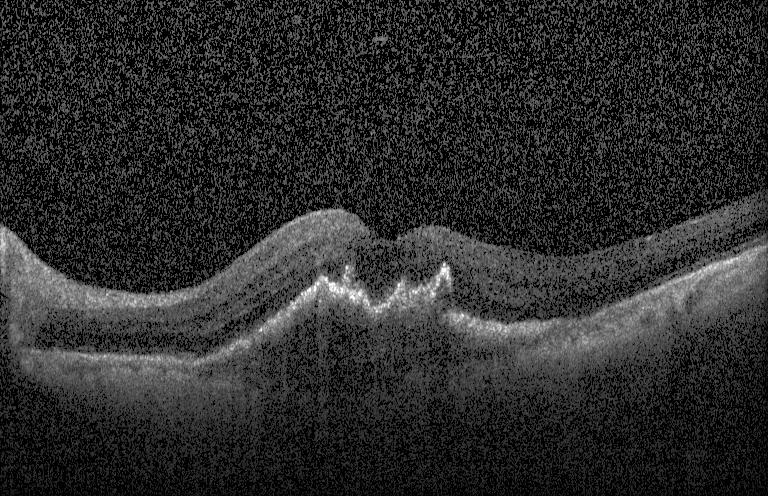

Macular OCT: a choroidal neovascular membrane.